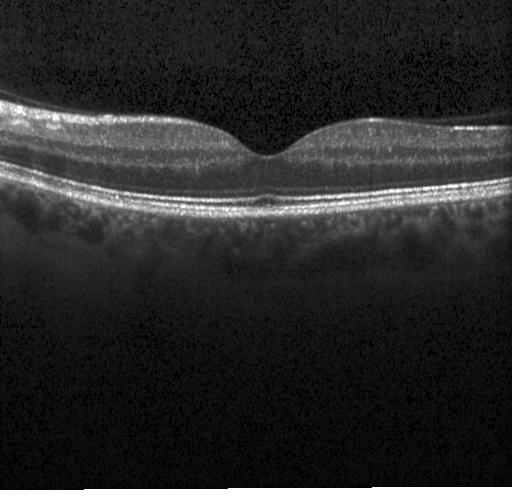
Retinal OCT B-scan
The scan shows no choroidal neovascularization, no diabetic macular edema, and no drusen.